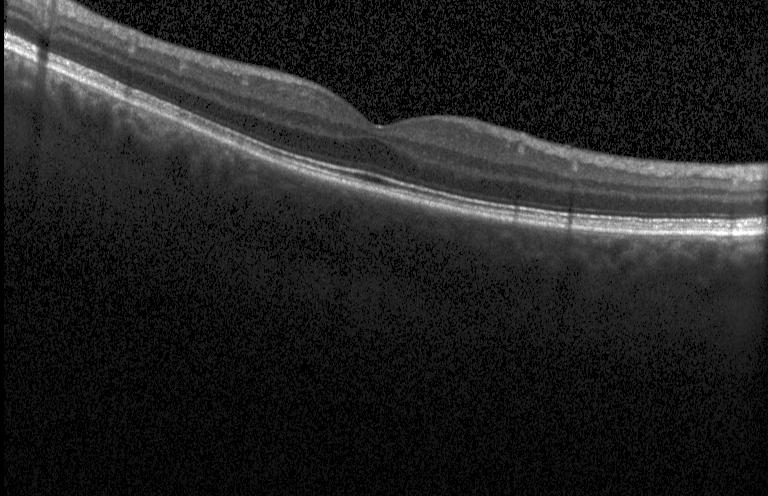 Retinal OCT cross-section showing no CNV, no DME, and no drusen.